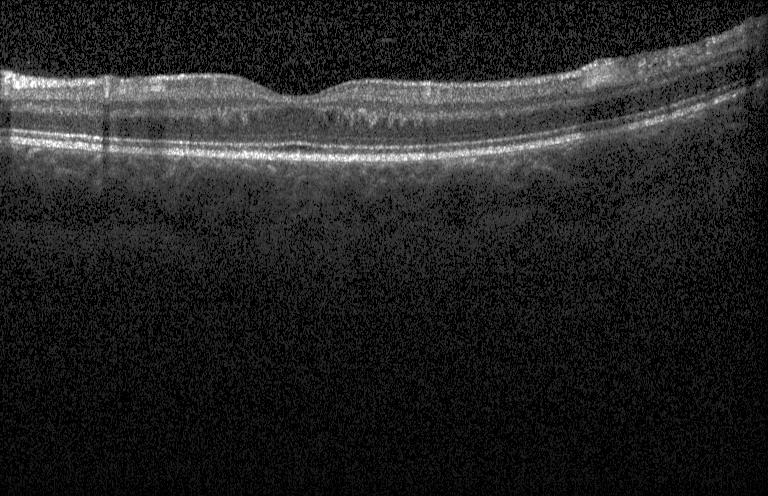 Finding: neither CNV, DME, nor drusen.